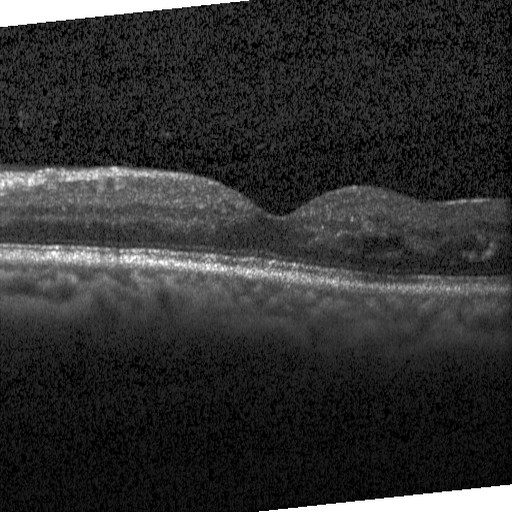

Through the macula, OCT line scan, instrument: Heidelberg Spectralis, spectral-domain optical coherence tomography — Finding: DME.